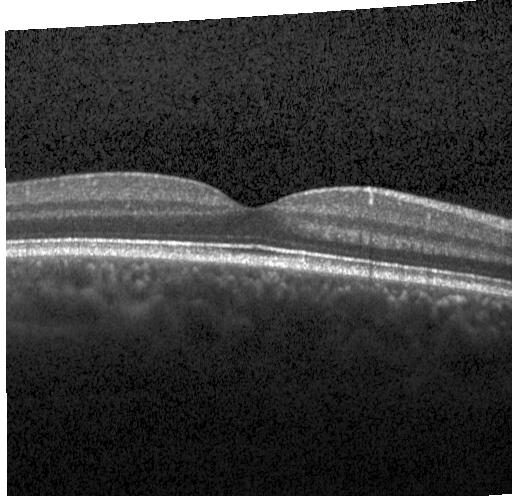

No choroidal neovascularization, no diabetic macular edema, and no drusen.